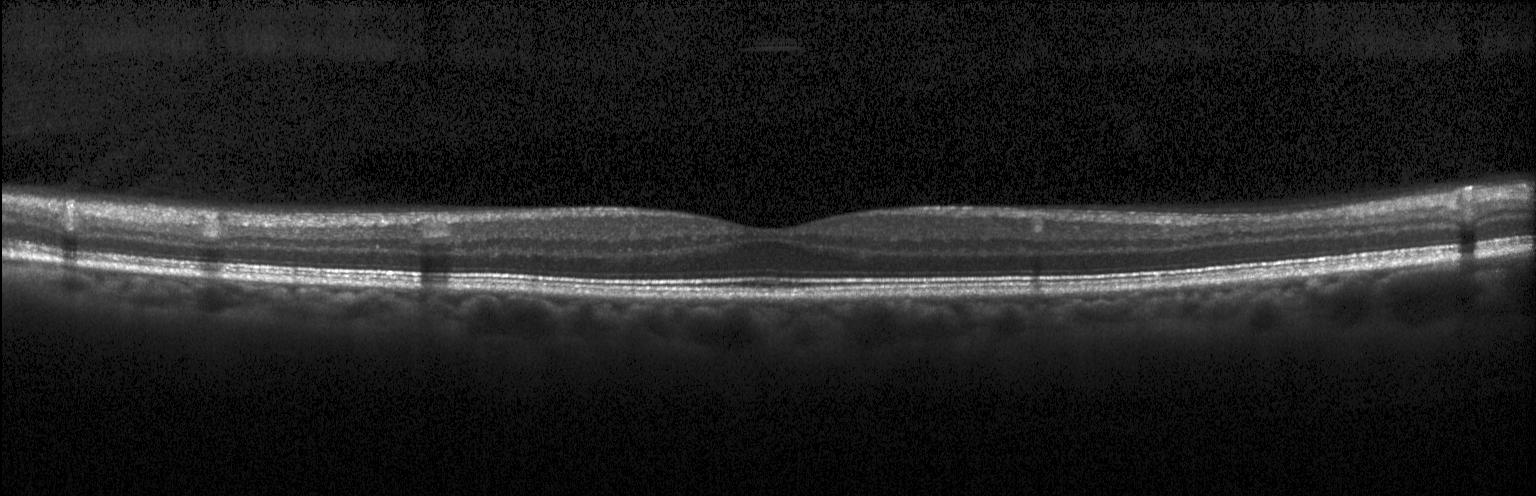

Acquired on a Heidelberg Spectralis, retinal OCT cross-section
Diagnosis: no evidence of CNV, DME, or drusen.